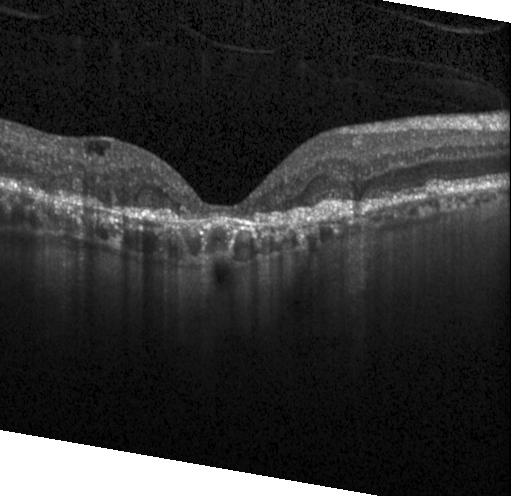

OCT B-scan, fovea-centered, spectral-domain OCT.
Macular OCT: a choroidal neovascular membrane.